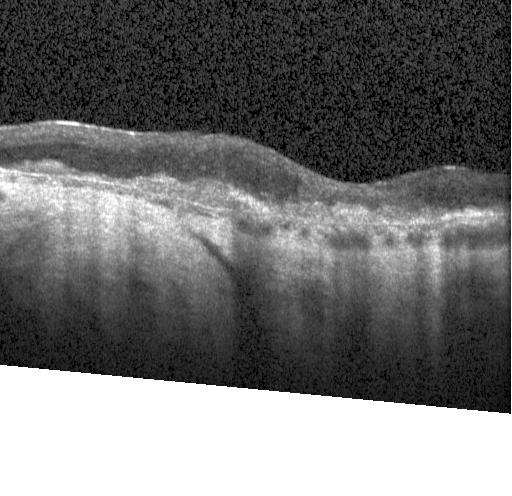 Retinal OCT B-scan. Finding: a choroidal neovascular membrane.